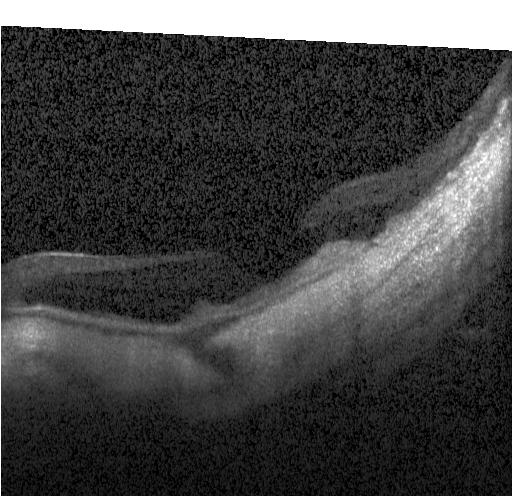 Acquired on a Heidelberg Spectralis, OCT line scan, macular scan.
Diagnosis: a choroidal neovascular membrane.